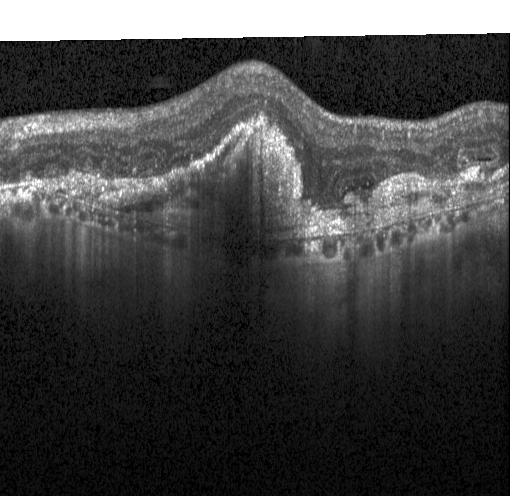

OCT B-scan
Diagnosis: a choroidal neovascular membrane.